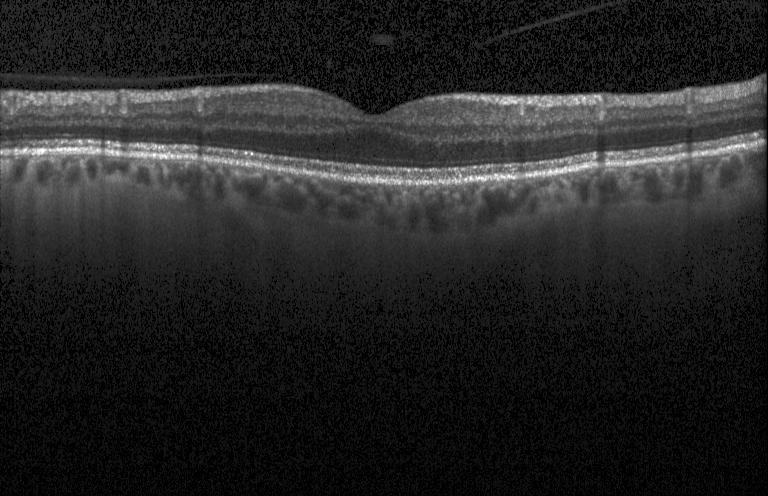
Horizontal scan through the fovea; optical coherence tomography scan. Diagnosis: no evidence of choroidal neovascularization, diabetic macular edema, or drusen.